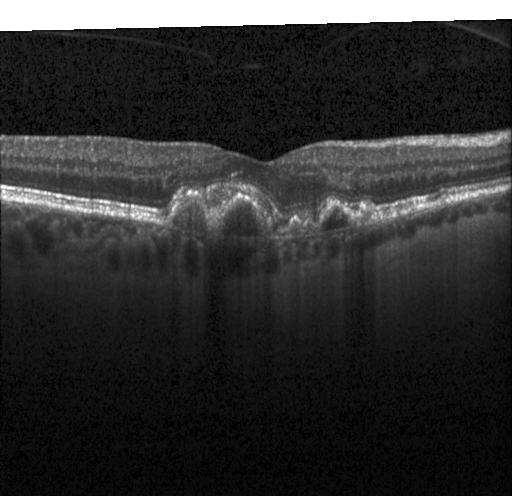
Spectral-domain optical coherence tomography. Heidelberg Spectralis OCT system. Retinal OCT B-scan — OCT finding: a choroidal neovascular membrane.